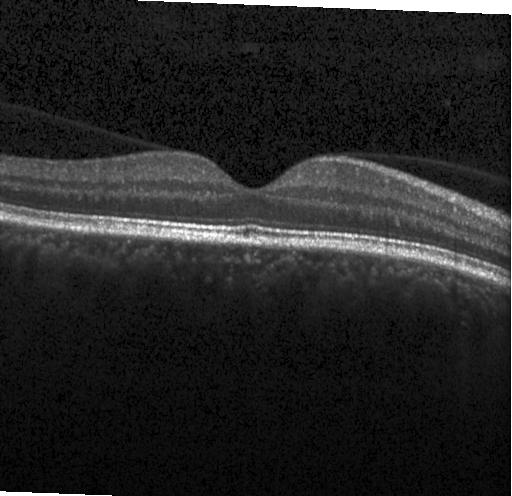
OCT finding: no choroidal neovascularization, diabetic macular edema, or drusen.